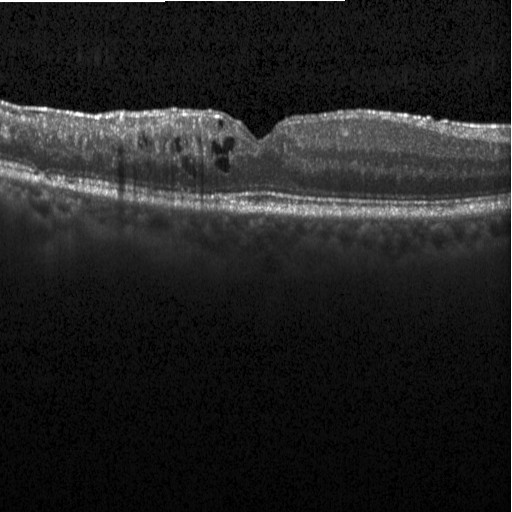

Retinal OCT cross-section · Heidelberg Spectralis OCT system · horizontal scan through the fovea.
This B-scan demonstrates diabetic macular edema (DME).